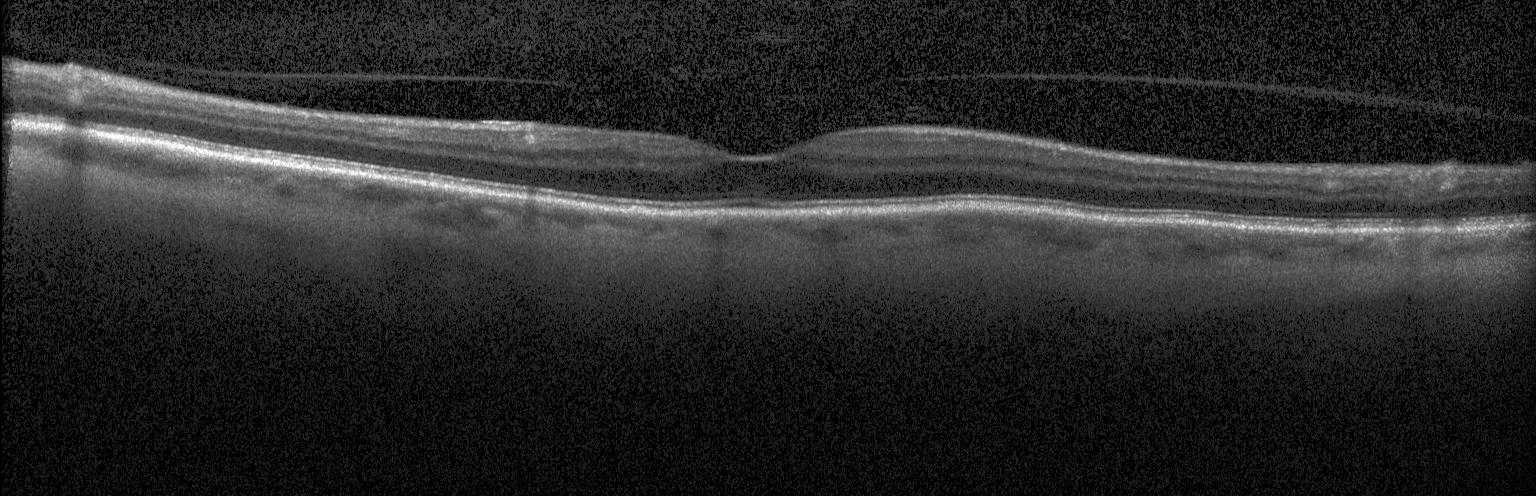 Finding: neither choroidal neovascularization, diabetic macular edema, nor drusen.